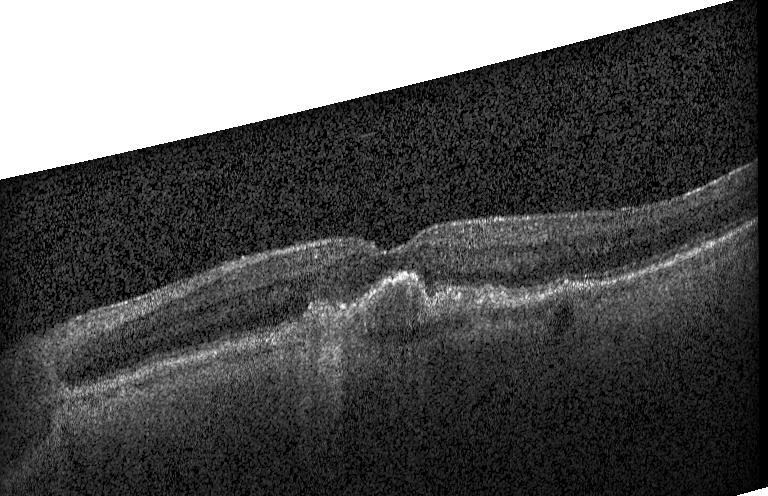

Through the macula. Heidelberg Spectralis OCT system. Retinal OCT cross-section. Spectral-domain OCT. The scan shows a choroidal neovascular membrane.